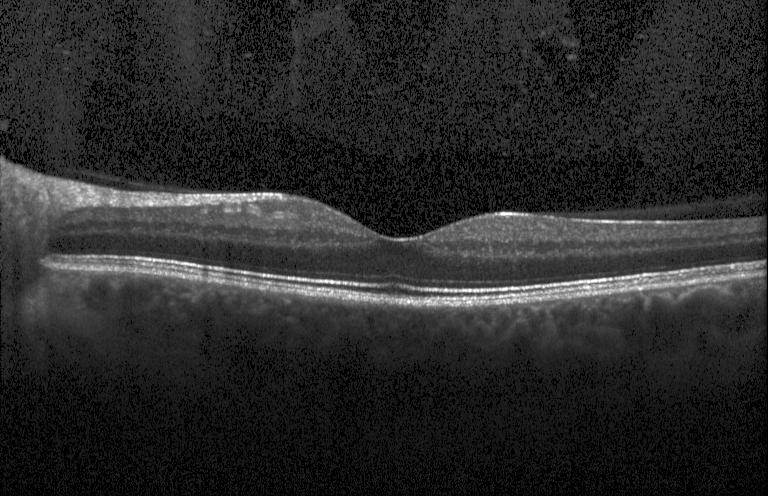

Macular scan · acquired on a Heidelberg Spectralis · optical coherence tomography B-scan. The scan shows no CNV, no DME, and no drusen.